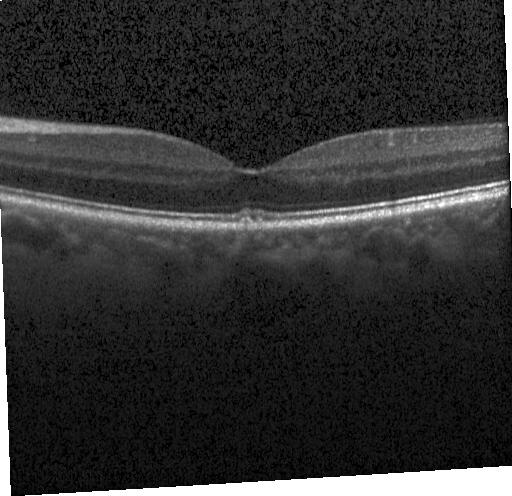
OCT finding: drusen.